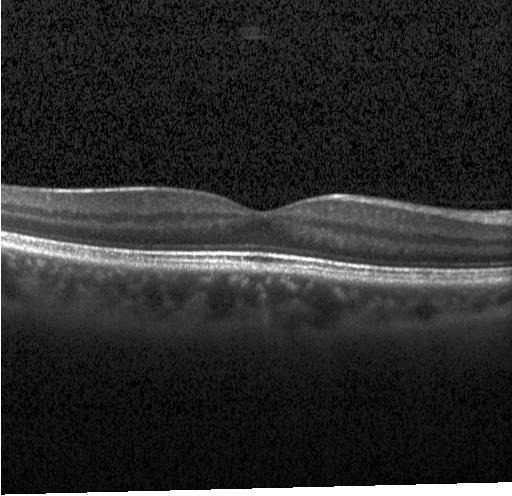
The scan shows no evidence of choroidal neovascularization, diabetic macular edema, or drusen.